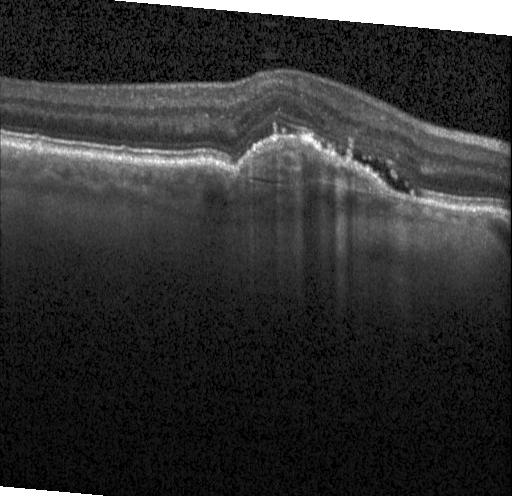
Instrument: Heidelberg Spectralis. Retinal OCT B-scan. Fovea-centered
Assessment: a choroidal neovascular membrane.